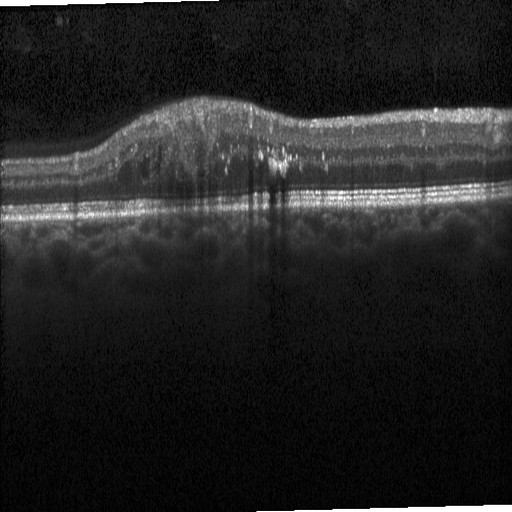
Spectral-domain optical coherence tomography · optical coherence tomography B-scan · instrument: Heidelberg Spectralis · through the macula. This B-scan demonstrates diabetic macular edema.